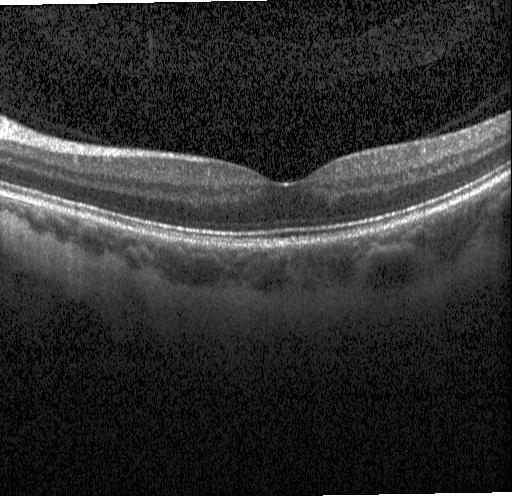

OCT B-scan; Heidelberg Spectralis; SD-OCT; centered on the fovea. Finding: no choroidal neovascularization, diabetic macular edema, or drusen.